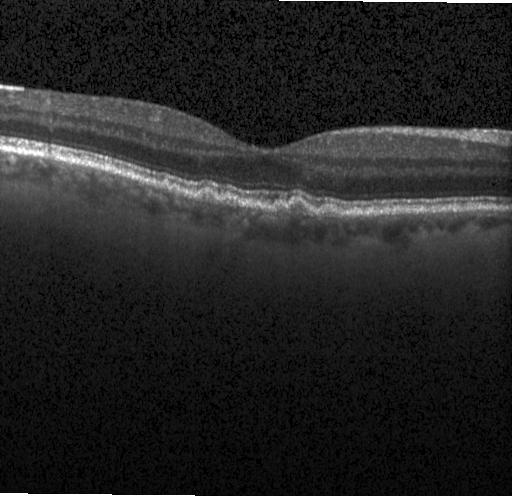

Optical coherence tomography scan; spectral-domain optical coherence tomography.
Assessment: sub-RPE drusenoid deposits.